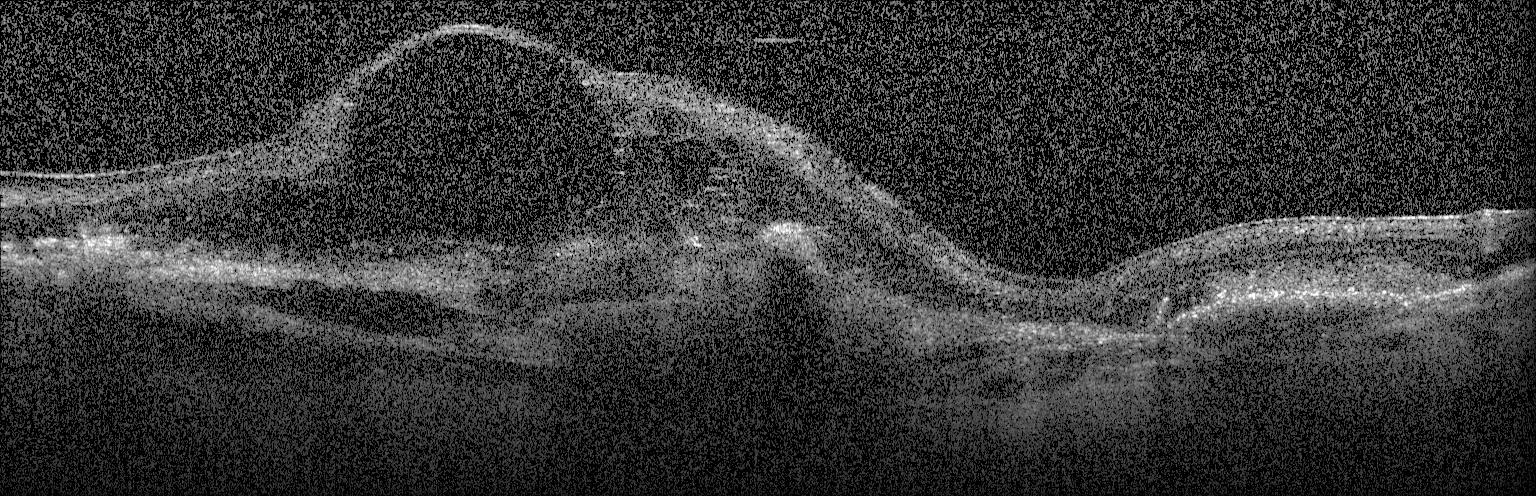
Retinal OCT cross-section. Impression: choroidal neovascularization (CNV).